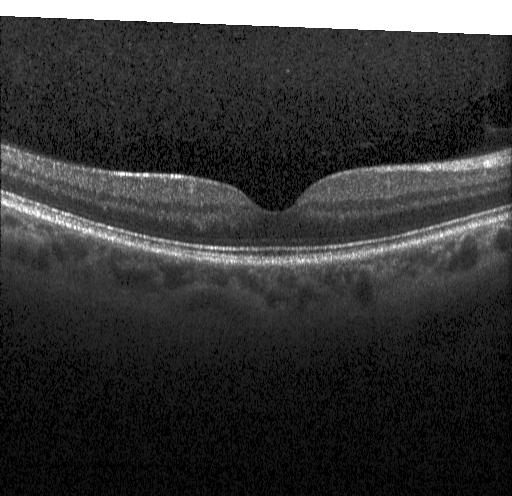 Retinal OCT cross-section showing no CNV, DME, or drusen.